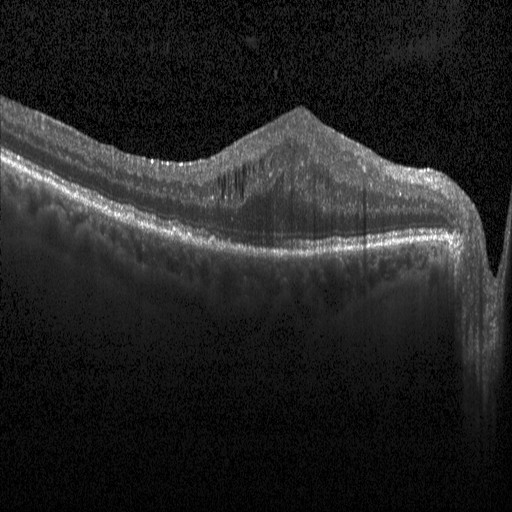
OCT finding: diabetic macular edema (DME).